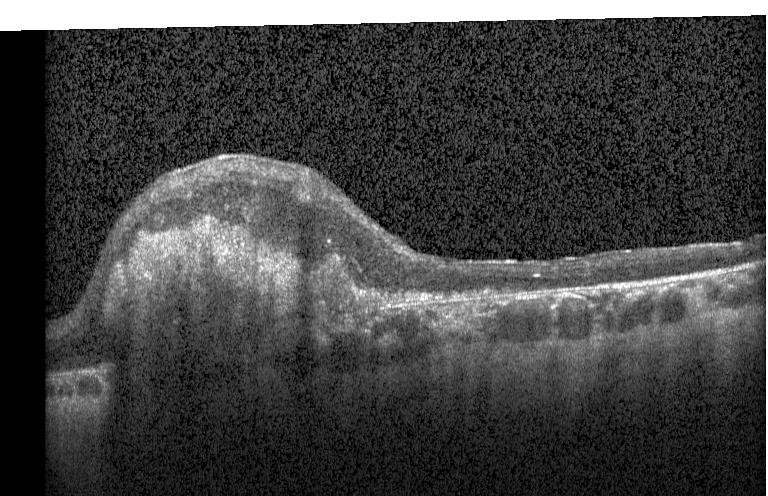 OCT B-scan. Diagnosis: choroidal neovascularization.